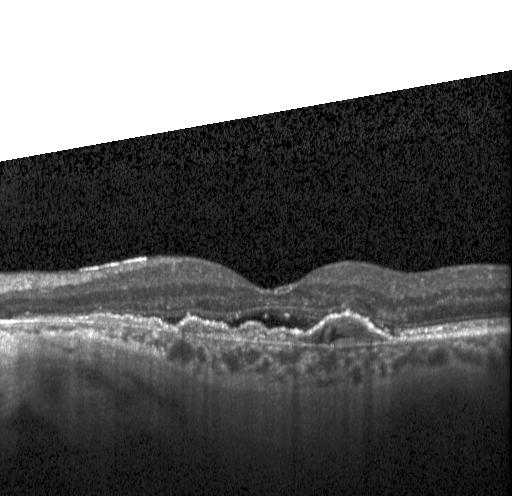 Retinal OCT cross-section; spectral-domain OCT; macular scan — Diagnosis: a choroidal neovascular membrane.